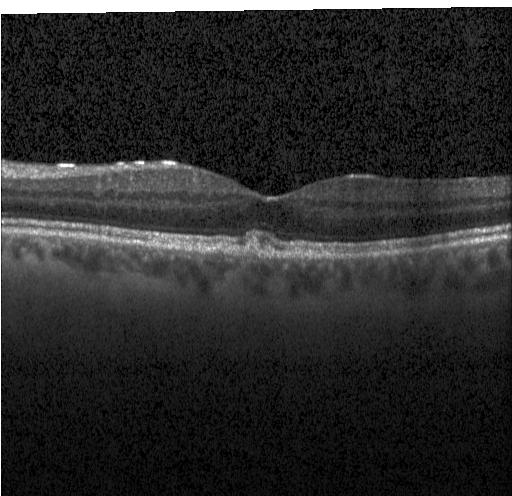
This B-scan demonstrates sub-RPE drusenoid deposits.